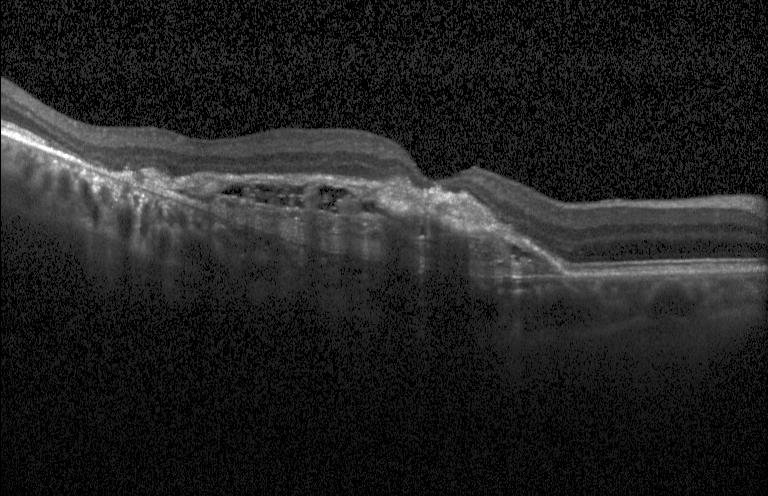

OCT B-scan
The scan shows a choroidal neovascular membrane.